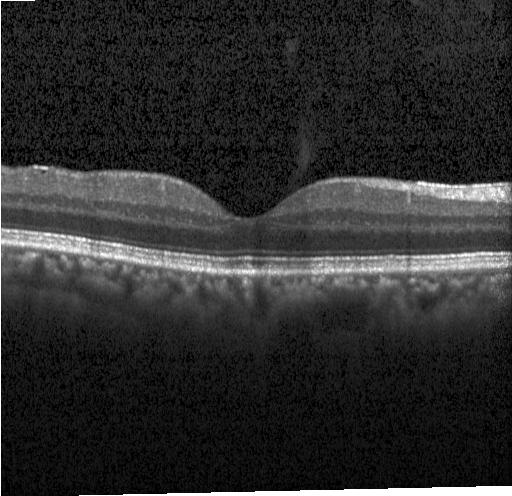 Macular scan · spectral-domain optical coherence tomography · optical coherence tomography B-scan
Macular OCT: no choroidal neovascularization, no diabetic macular edema, and no drusen.